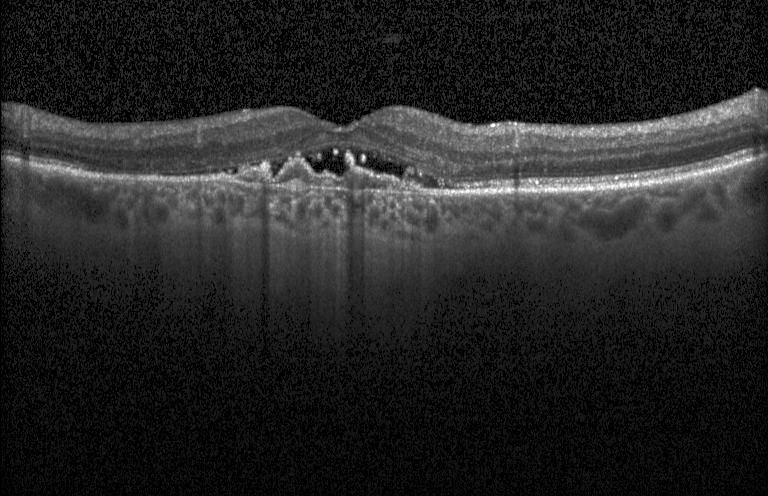 Spectral-domain OCT; macular scan; OCT B-scan — Diagnosis: a choroidal neovascular membrane.